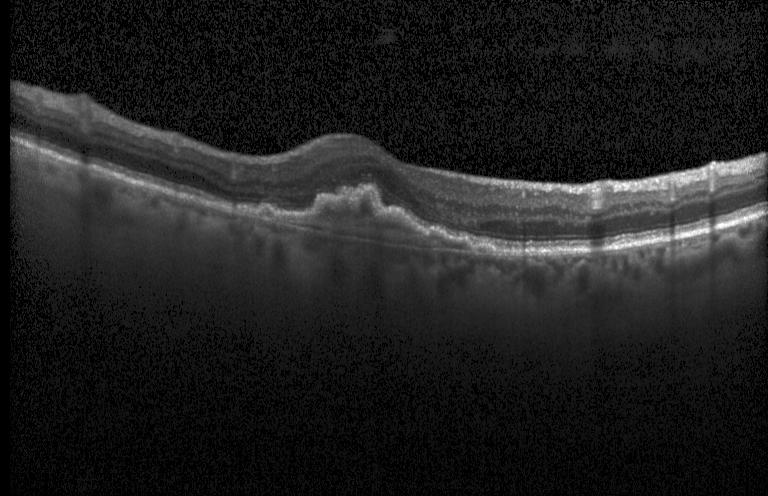 OCT line scan, SD-OCT.
Dx: a choroidal neovascular membrane.